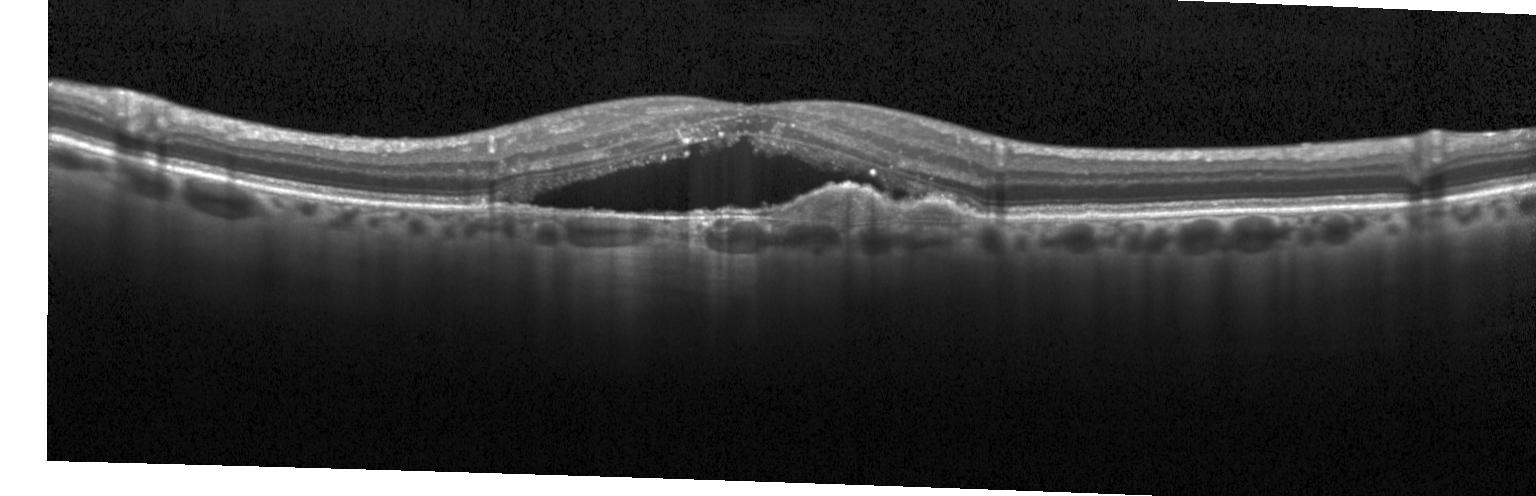
Finding: choroidal neovascularization (CNV).